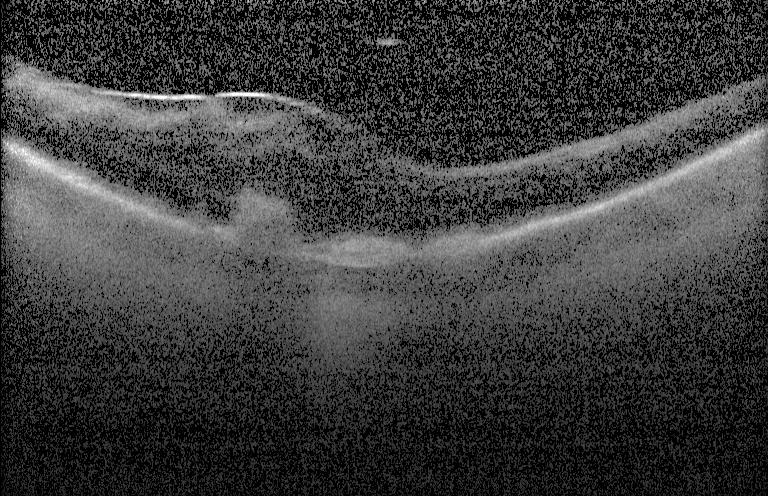
Assessment: CNV.